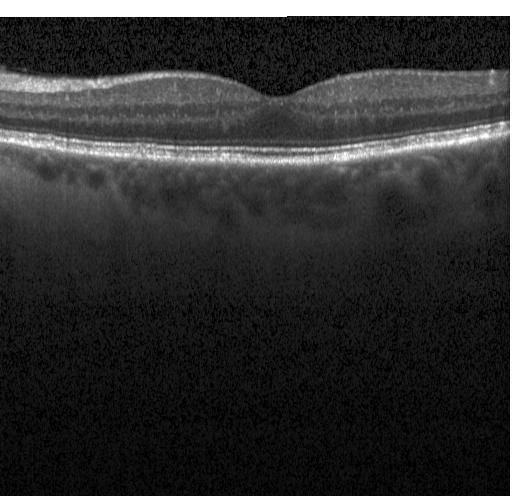
Retinal OCT B-scan; through the macula; Heidelberg Spectralis; SD-OCT
This B-scan demonstrates no choroidal neovascularization, no diabetic macular edema, and no drusen.